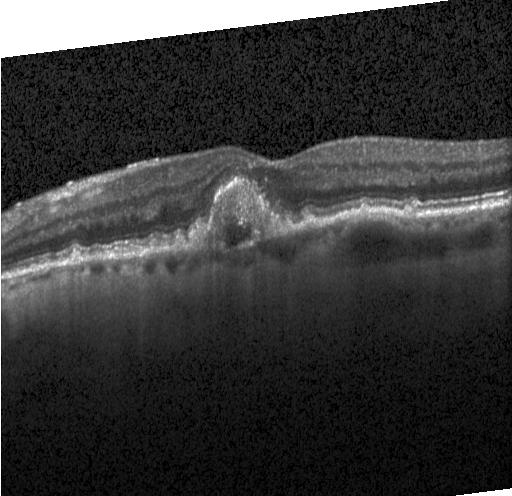
Dx: a choroidal neovascular membrane.